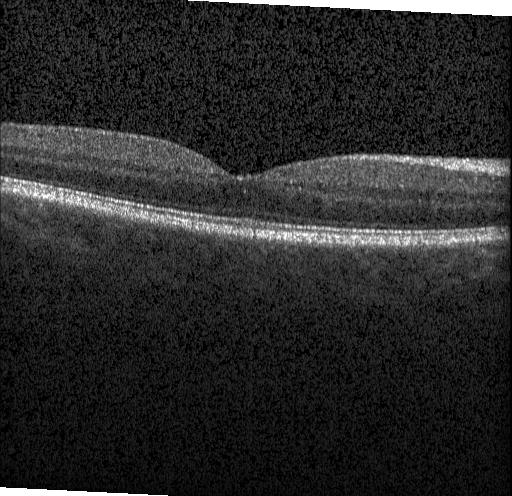
OCT line scan — Diagnosis: no choroidal neovascularization, no diabetic macular edema, and no drusen.